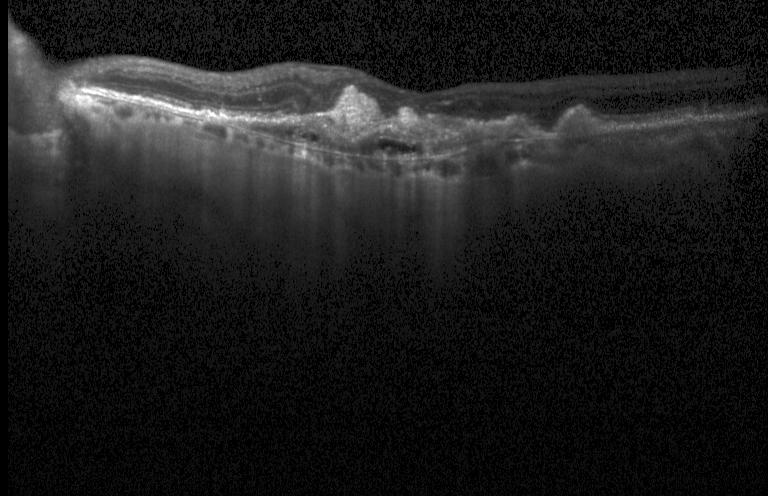

This B-scan demonstrates a choroidal neovascular membrane.